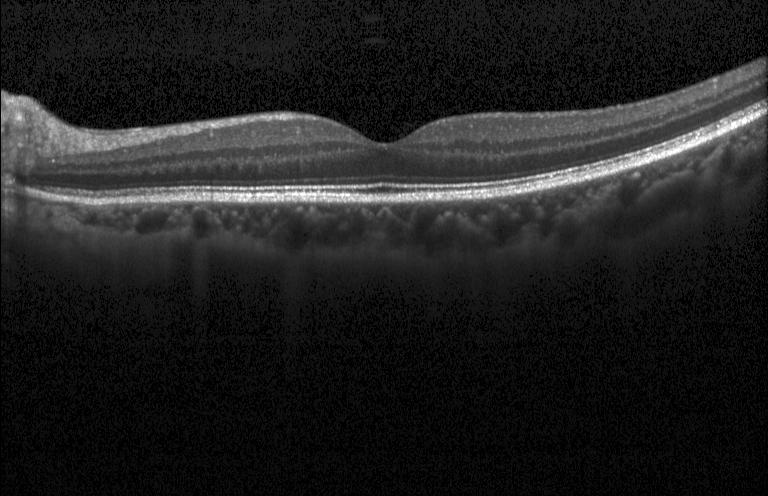 Through the macula. Acquired on a Heidelberg Spectralis. Optical coherence tomography B-scan. Spectral-domain optical coherence tomography — Diagnosis: no choroidal neovascularization, no diabetic macular edema, and no drusen.